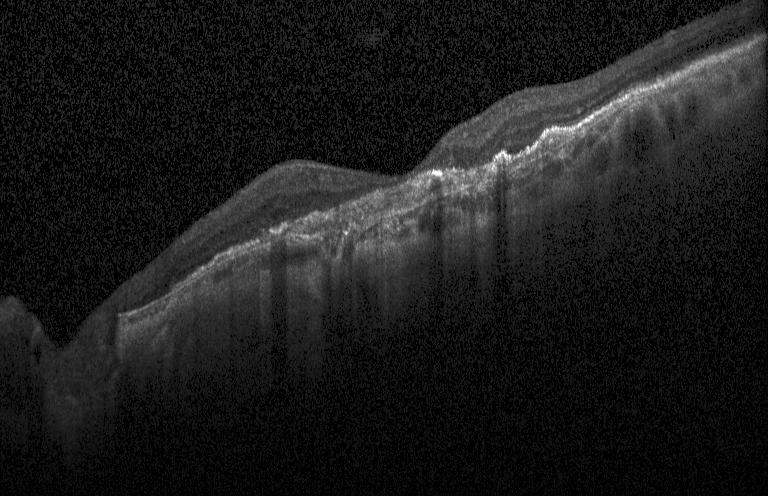

Retinal OCT cross-section; macular scan. Dx: choroidal neovascularization (CNV).